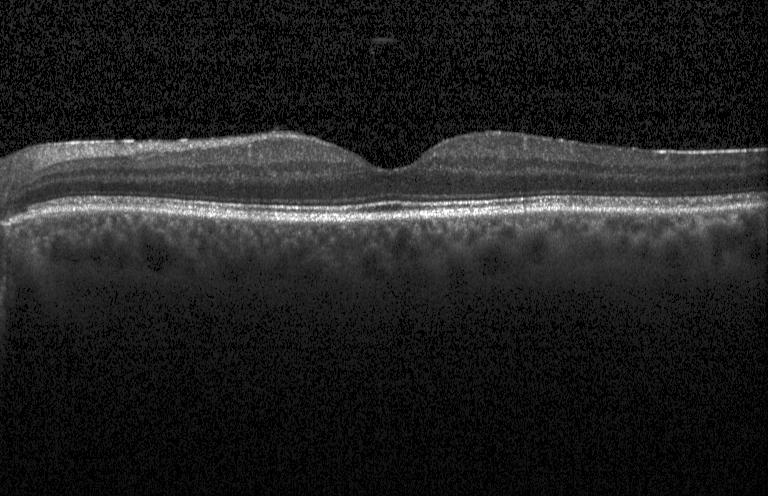 Retinal OCT B-scan. Spectral-domain optical coherence tomography. Instrument: Heidelberg Spectralis
Assessment: no CNV, DME, or drusen.